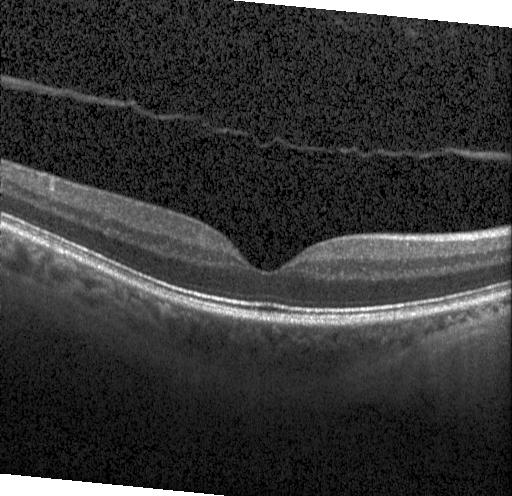 Spectral-domain optical coherence tomography · retinal OCT cross-section. OCT finding: no CNV, DME, or drusen.